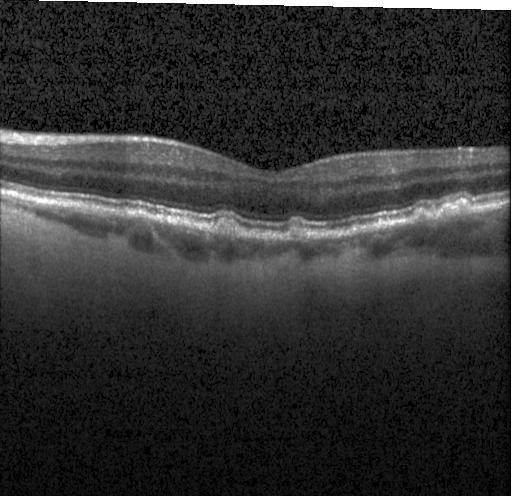
Impression: sub-RPE drusenoid deposits.